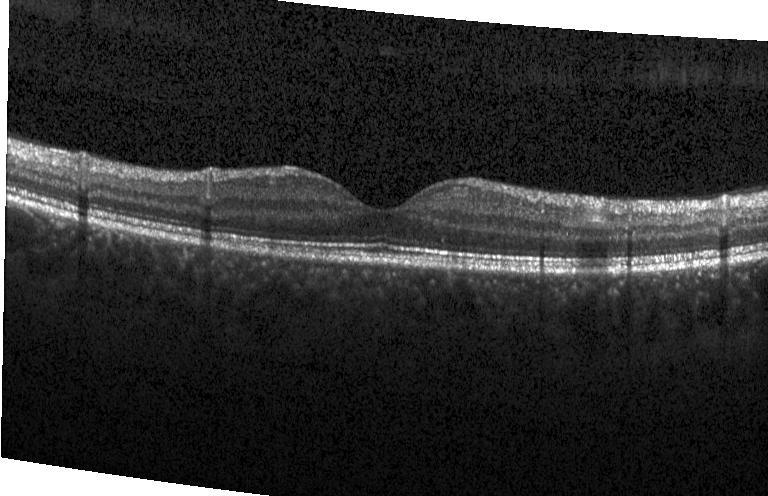
Retinal OCT B-scan. Through the macula. Impression: no choroidal neovascularization, diabetic macular edema, or drusen.